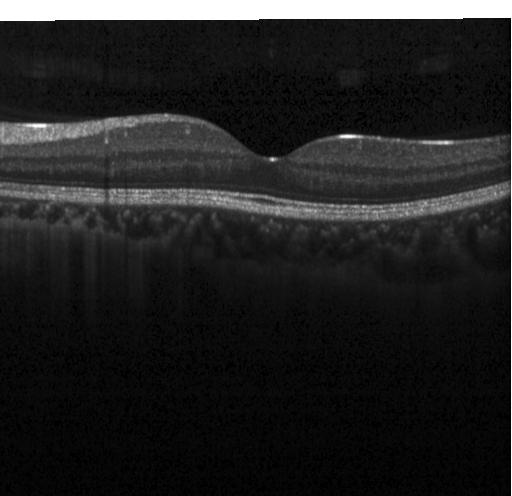

Finding: no choroidal neovascularization, diabetic macular edema, or drusen.